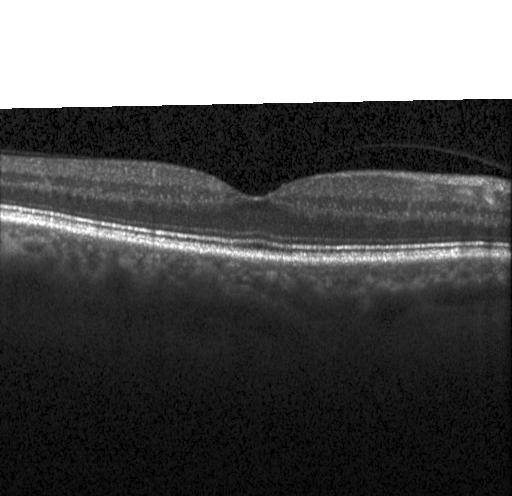
Acquired on a Heidelberg Spectralis. Optical coherence tomography B-scan. Macular scan.
Dx: no evidence of CNV, DME, or drusen.